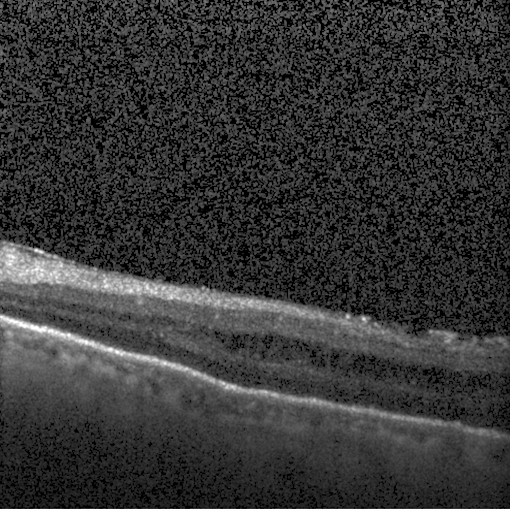 OCT finding: DME.